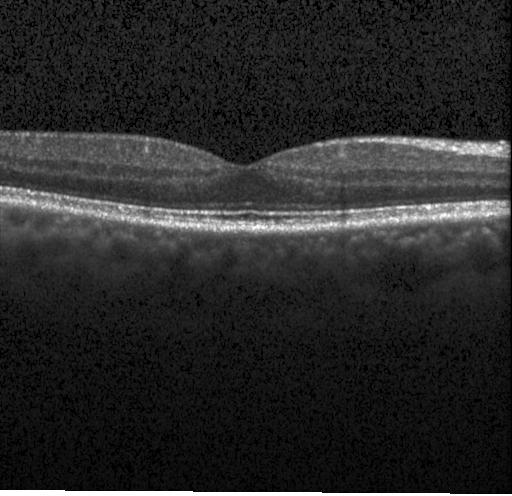
Dx: no evidence of CNV, DME, or drusen.